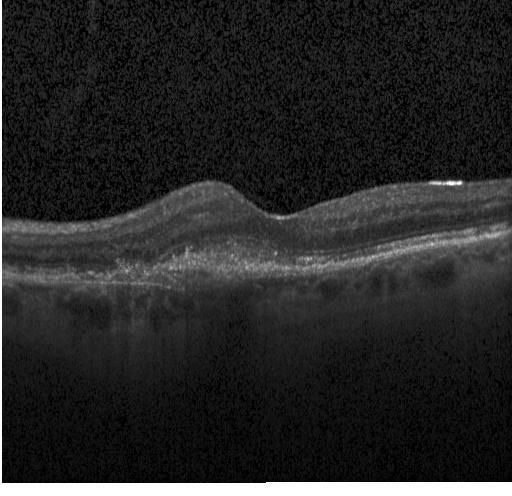 Spectral-domain OCT B-scan: choroidal neovascularization (CNV).